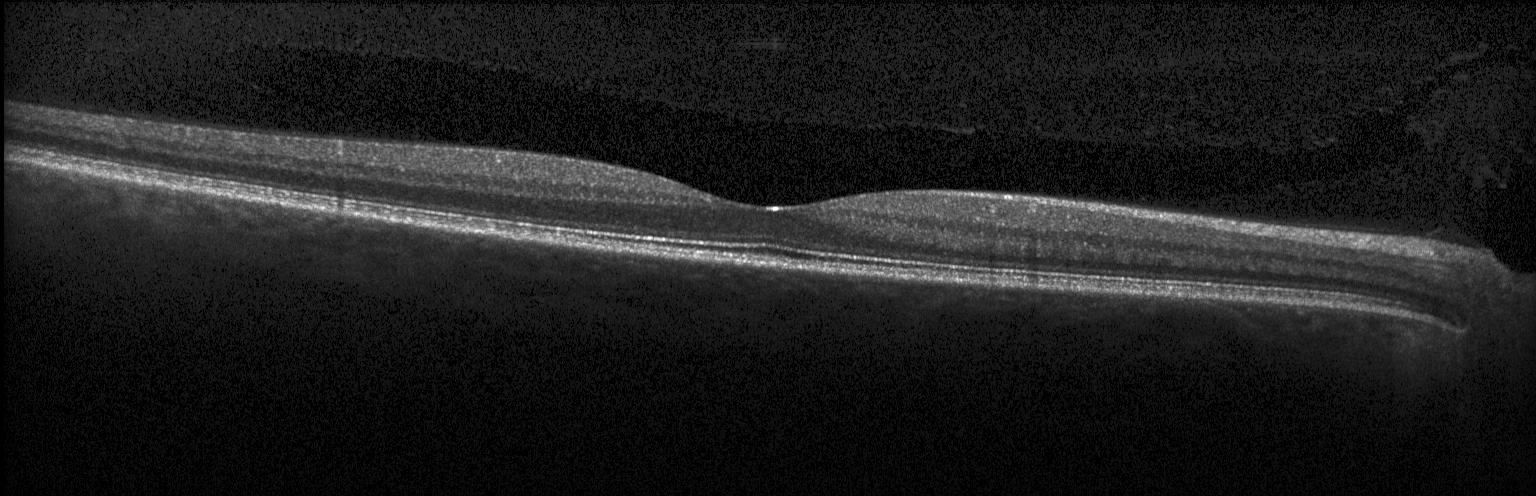

OCT line scan · spectral-domain OCT — Assessment: no CNV, DME, or drusen.